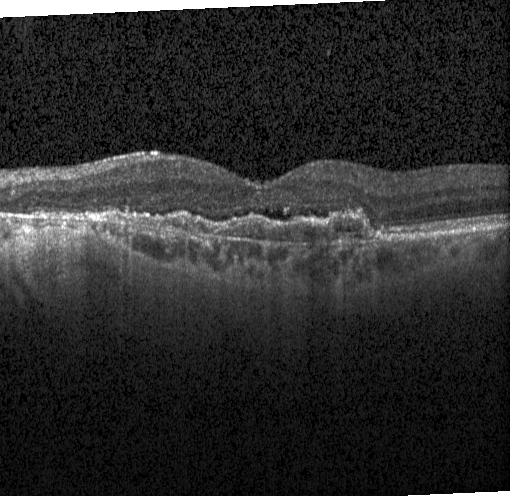

OCT finding: a choroidal neovascular membrane.